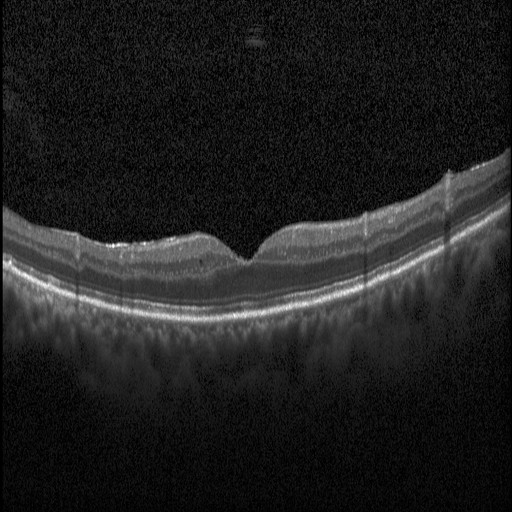

OCT finding: DME.